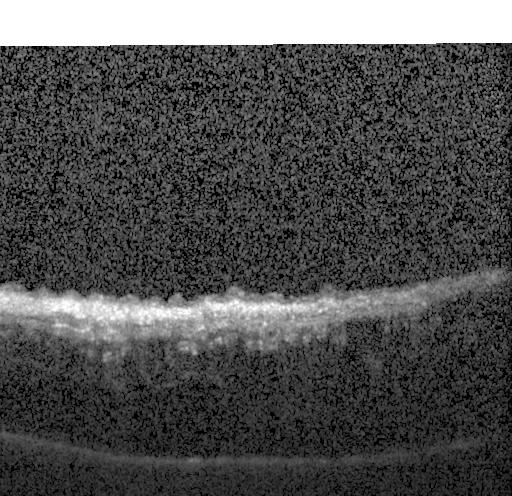 Optical coherence tomography scan
Assessment: diabetic macular edema (DME).